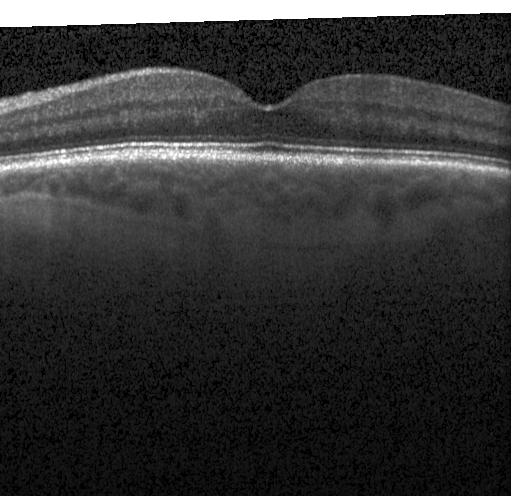

OCT line scan.
Finding: no CNV, DME, or drusen.